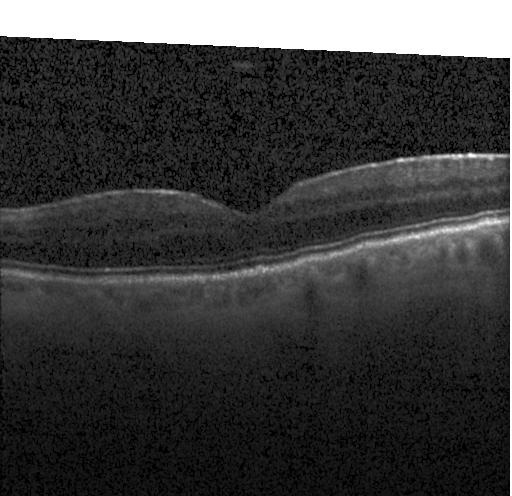

OCT B-scan, spectral-domain OCT. Finding: no evidence of choroidal neovascularization, diabetic macular edema, or drusen.